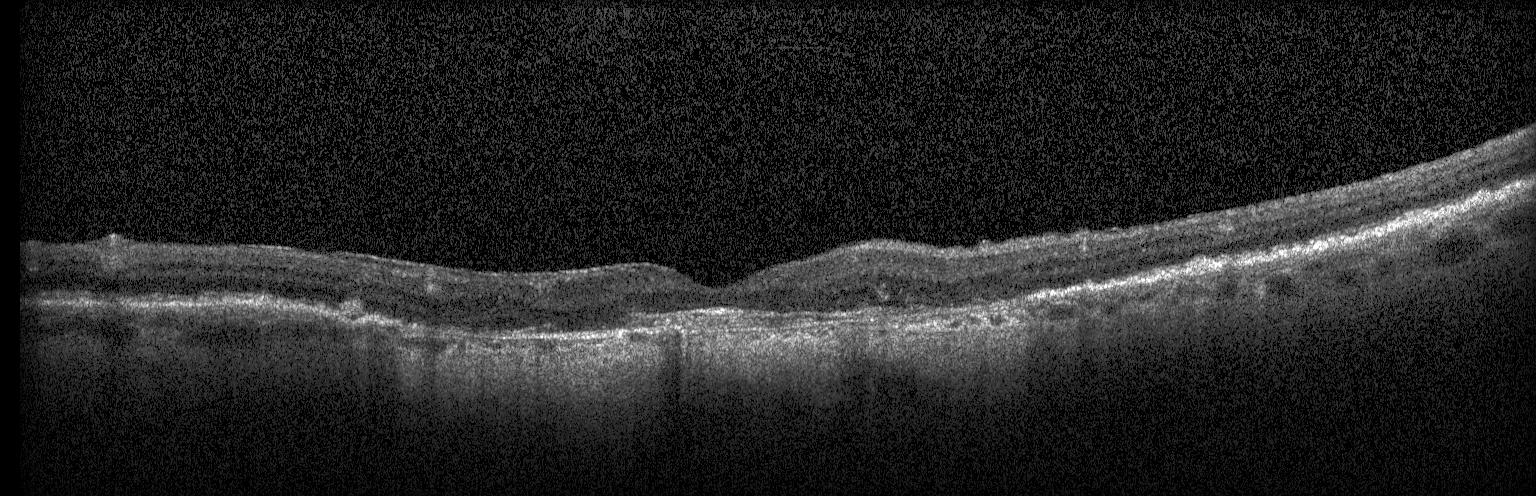 Dx: choroidal neovascularization.